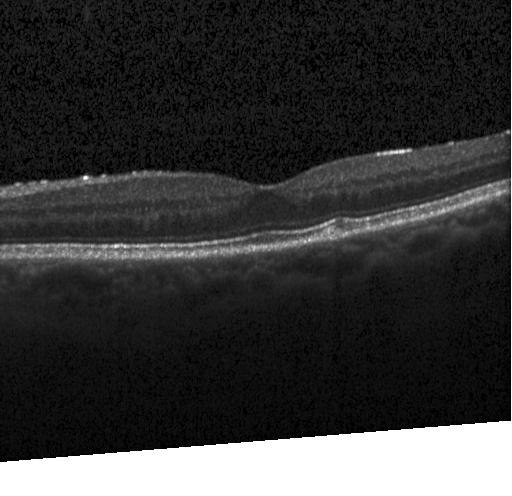

Heidelberg Spectralis OCT system. Centered on the fovea. Retinal OCT B-scan. Assessment: no CNV, no DME, and no drusen.